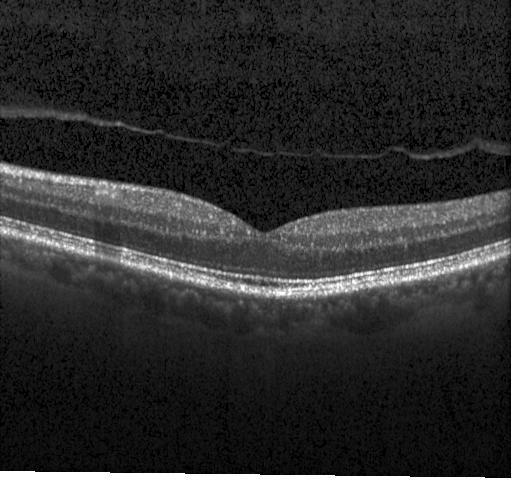
OCT scan showing neither choroidal neovascularization, diabetic macular edema, nor drusen.